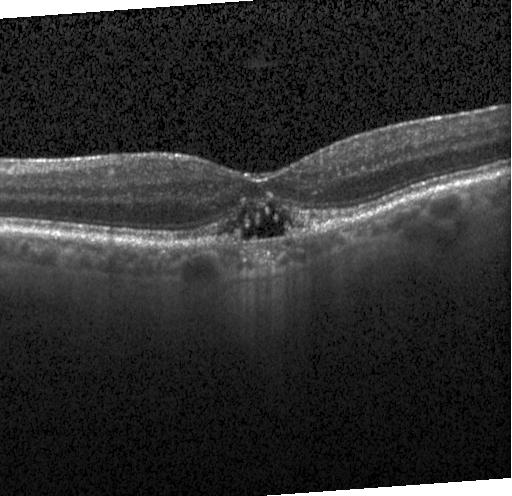
Retinal OCT cross-section; Heidelberg Spectralis OCT system; spectral-domain OCT; centered on the fovea — Diagnosis: a choroidal neovascular membrane.